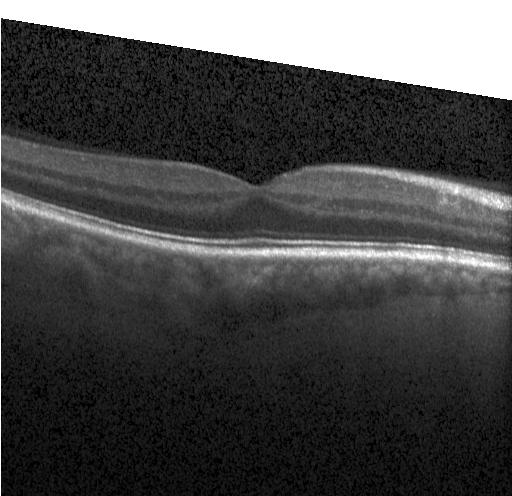 Spectral-domain optical coherence tomography. Instrument: Heidelberg Spectralis. Macular scan. OCT line scan
This B-scan demonstrates no choroidal neovascularization, no diabetic macular edema, and no drusen.